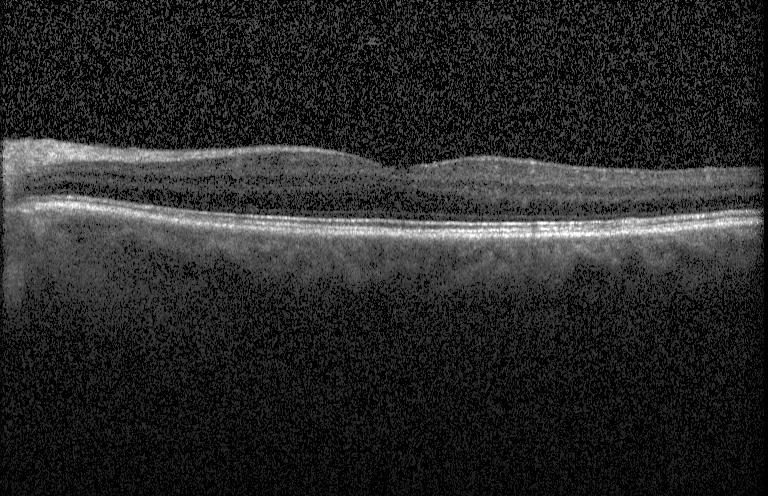 Retinal OCT cross-section.
Diagnosis: neither CNV, DME, nor drusen.